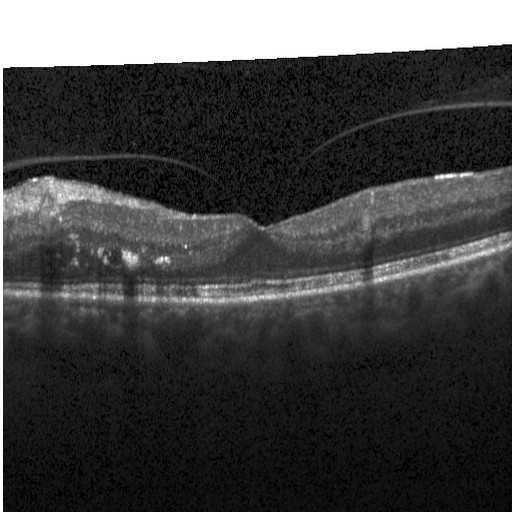
SD-OCT · optical coherence tomography B-scan · instrument: Heidelberg Spectralis — This B-scan demonstrates diabetic macular edema.